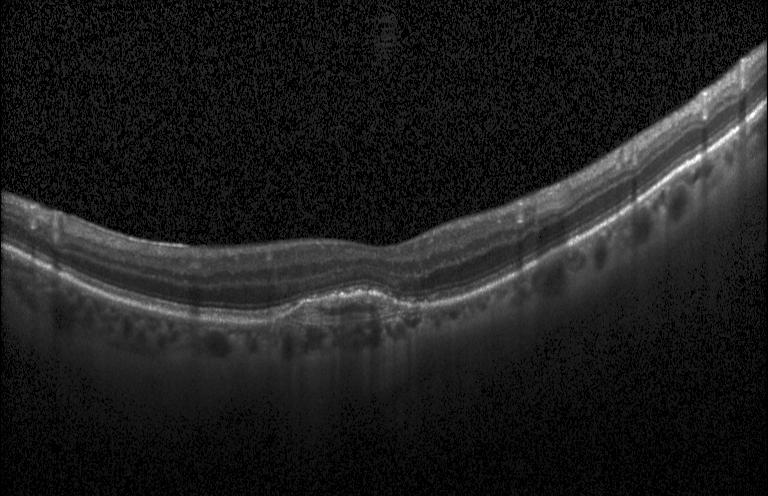
Retinal OCT cross-section. The scan shows a choroidal neovascular membrane.